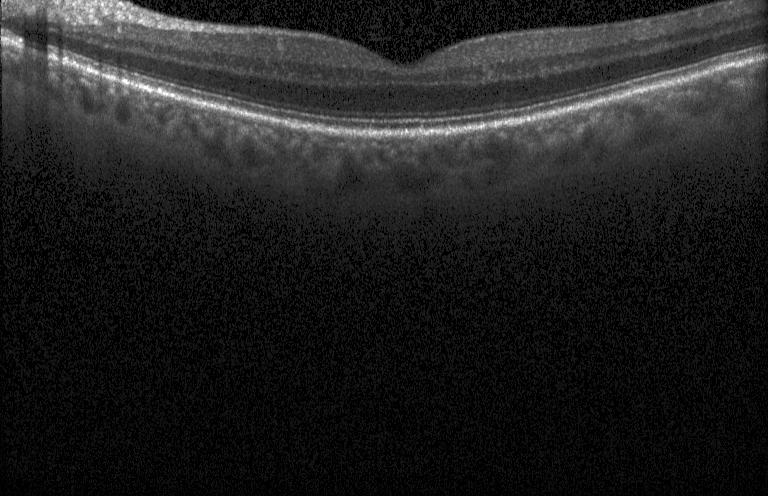 Heidelberg Spectralis OCT system. Retinal OCT B-scan.
Finding: no choroidal neovascularization, diabetic macular edema, or drusen.